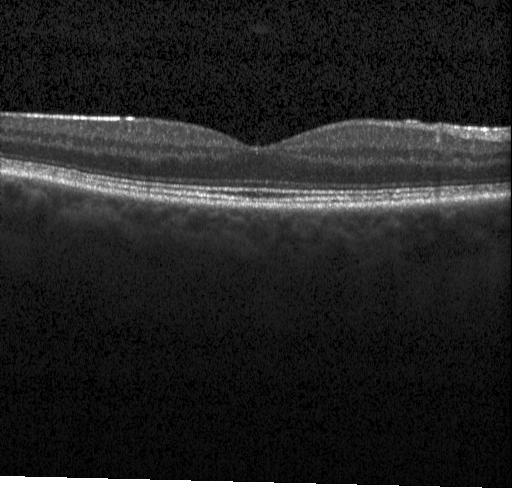 Finding: no CNV, no DME, and no drusen.